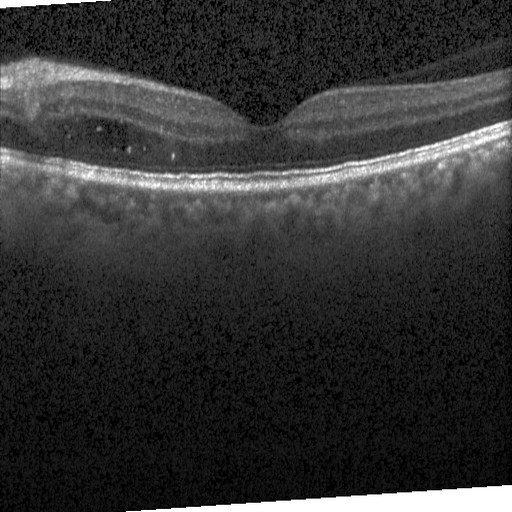
OCT line scan.
Diagnosis: DME.